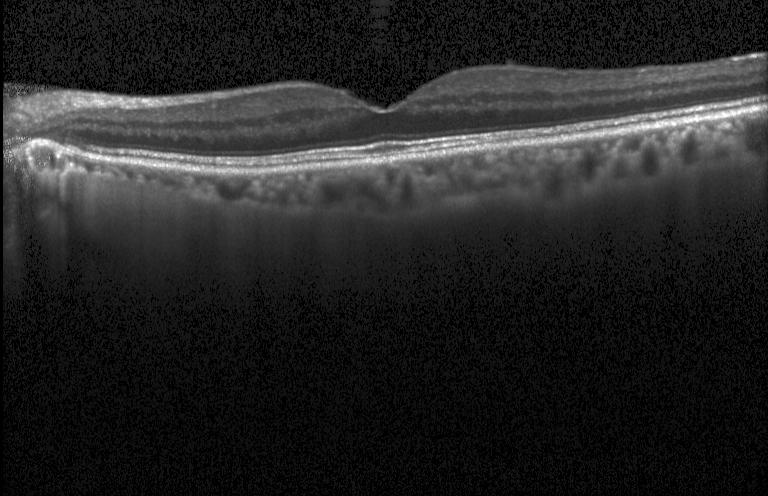
Acquired on a Heidelberg Spectralis. OCT line scan. Macular scan
OCT finding: no choroidal neovascularization, diabetic macular edema, or drusen.